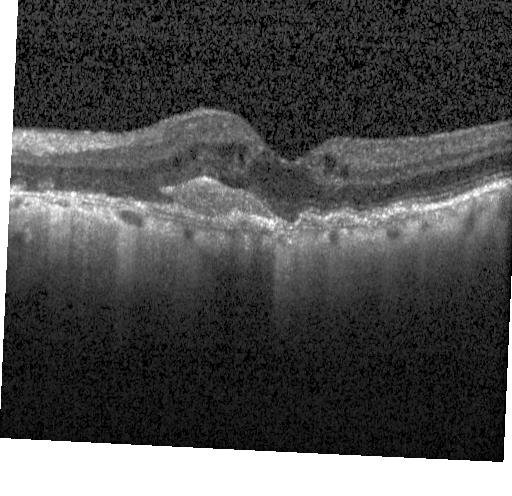

This B-scan demonstrates a choroidal neovascular membrane.